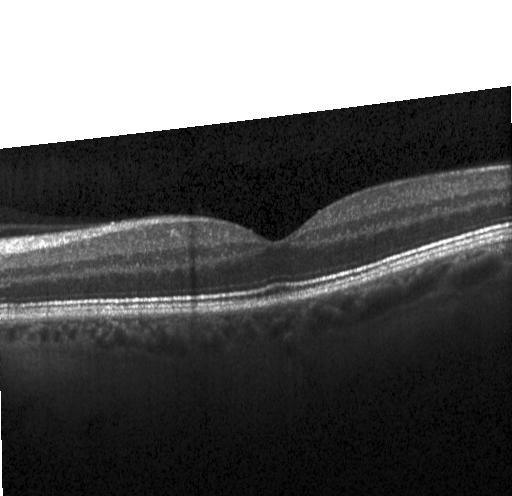 Spectral-domain OCT. Heidelberg Spectralis. Optical coherence tomography B-scan.
Impression: no evidence of CNV, DME, or drusen.